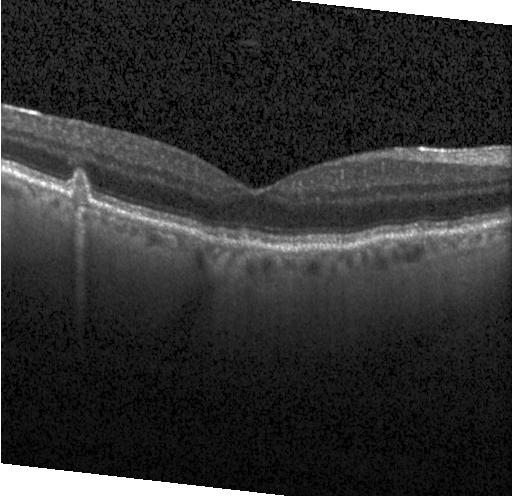

Impression: drusen.